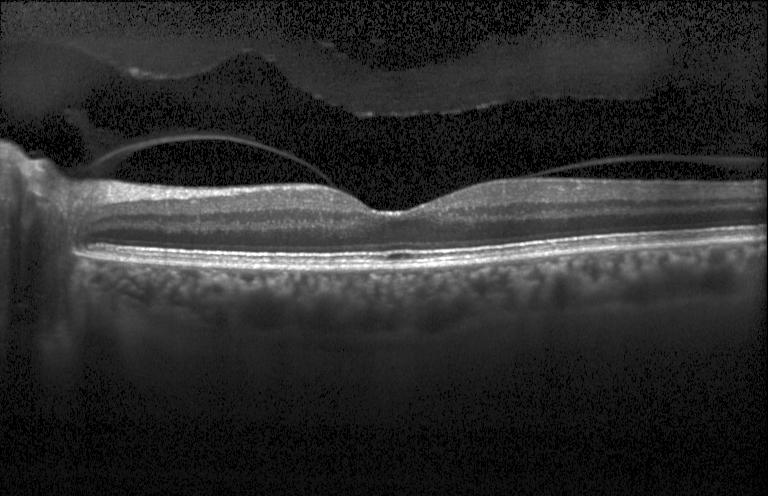 OCT B-scan — Diagnosis: no CNV, DME, or drusen.